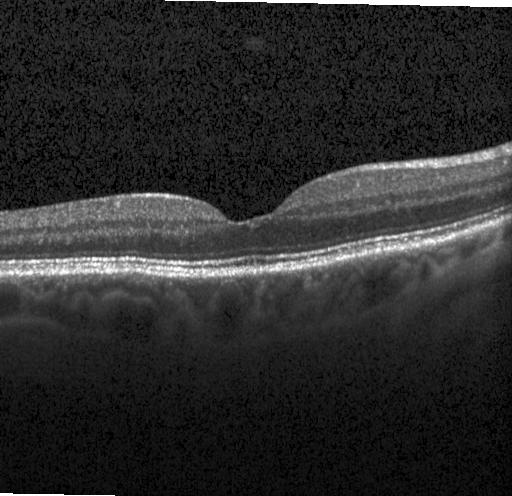

Optical coherence tomography scan; fovea-centered
Finding: neither CNV, DME, nor drusen.